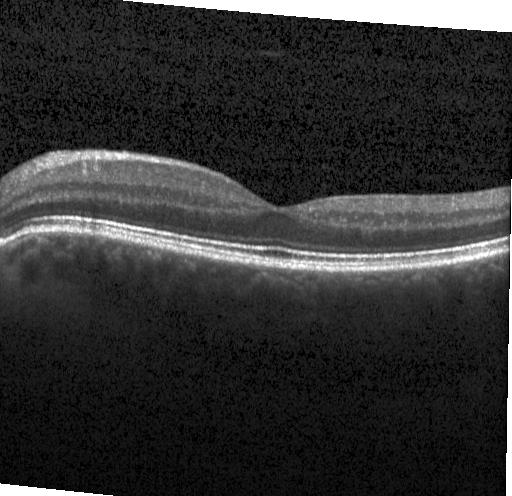

SD-OCT; optical coherence tomography B-scan; Heidelberg Spectralis; centered on the fovea — Diagnosis: neither choroidal neovascularization, diabetic macular edema, nor drusen.